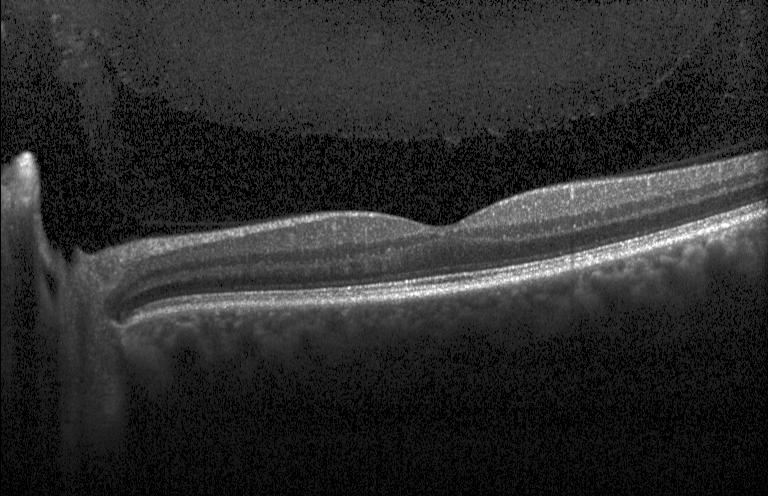
Instrument: Heidelberg Spectralis; through the macula; SD-OCT; retinal OCT B-scan
OCT finding: no choroidal neovascularization, no diabetic macular edema, and no drusen.